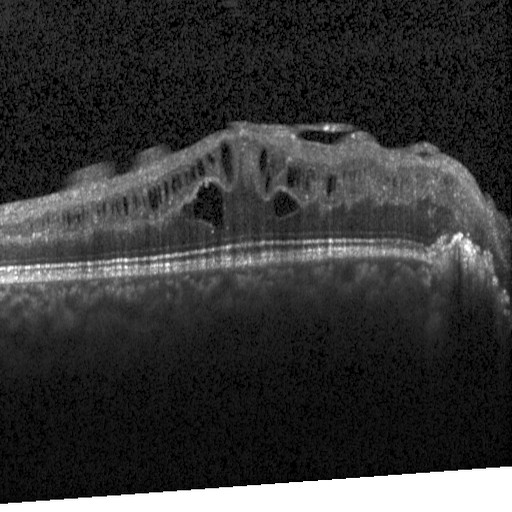

OCT line scan. Acquired on a Heidelberg Spectralis
Diagnosis: DME.